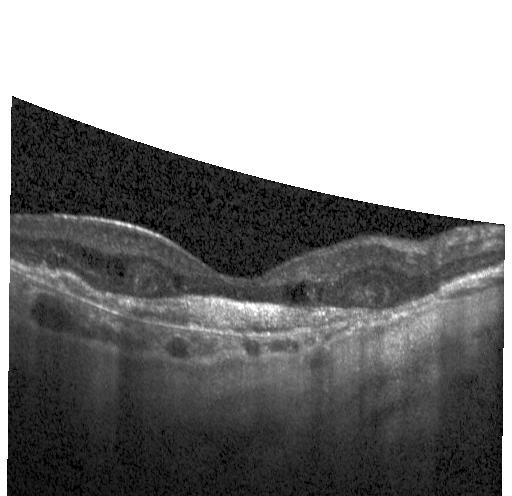
OCT line scan · horizontal scan through the fovea · spectral-domain OCT · acquired on a Heidelberg Spectralis. OCT finding: a choroidal neovascular membrane.